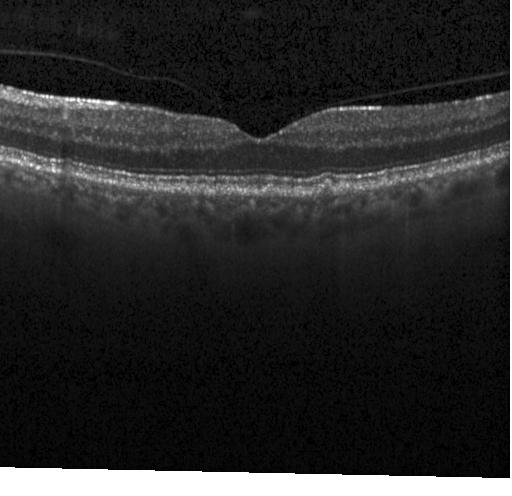

OCT B-scan; centered on the fovea — Finding: drusen.